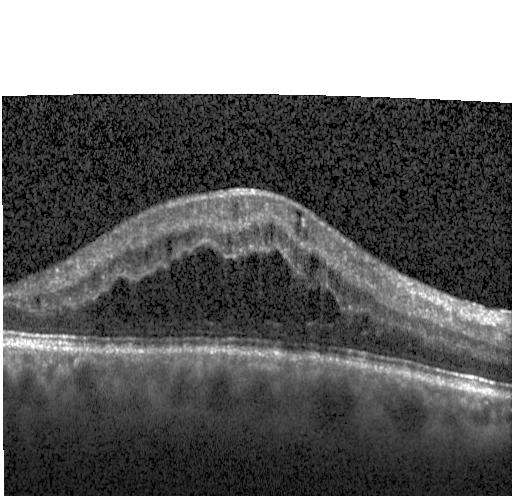 Retinal OCT cross-section. Spectral-domain optical coherence tomography. Heidelberg Spectralis OCT system. Macular scan. Impression: diabetic macular edema.